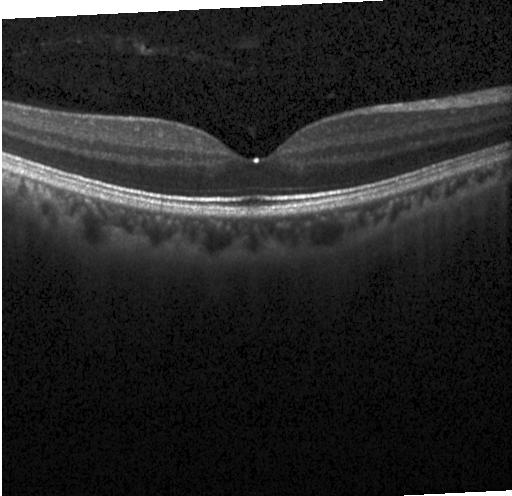
Retinal OCT cross-section. Macular scan. Acquired on a Heidelberg Spectralis — The scan shows no choroidal neovascularization, no diabetic macular edema, and no drusen.